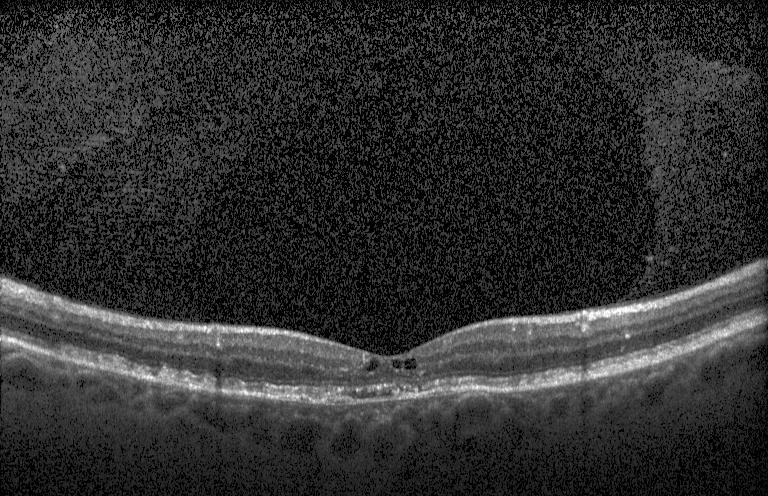
Macular OCT demonstrating a choroidal neovascular membrane.